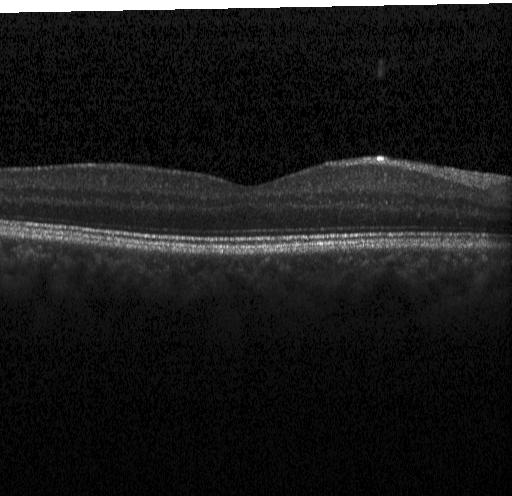

Spectral-domain optical coherence tomography · macular scan · OCT B-scan · instrument: Heidelberg Spectralis.
Dx: neither CNV, DME, nor drusen.